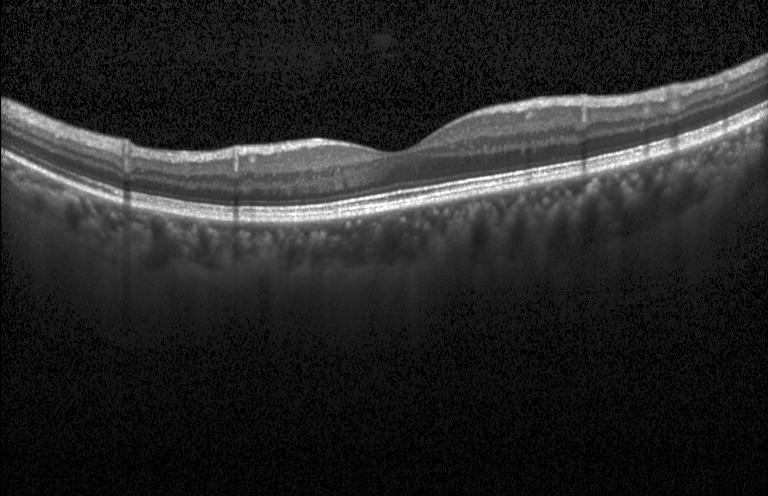

Retinal OCT B-scan
Finding: no evidence of CNV, DME, or drusen.